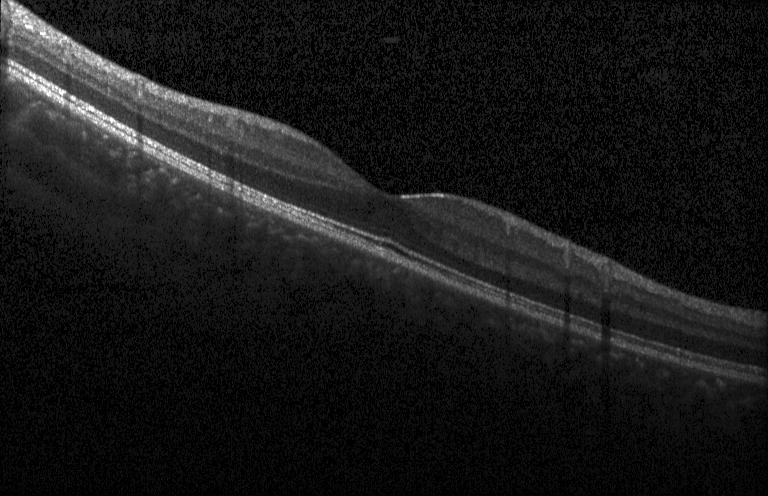
Heidelberg Spectralis; retinal OCT B-scan.
Finding: no CNV, no DME, and no drusen.